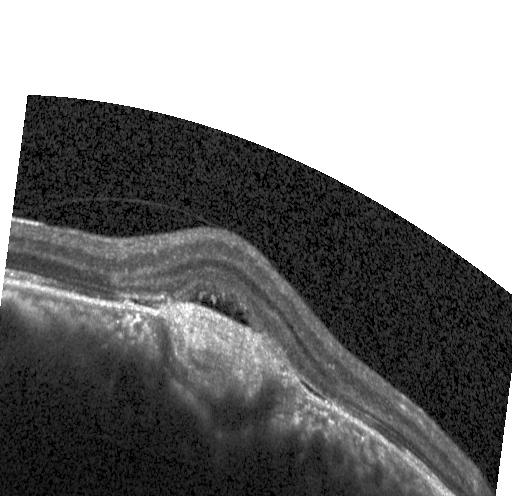
Optical coherence tomography B-scan. Spectral-domain optical coherence tomography.
Finding: CNV.